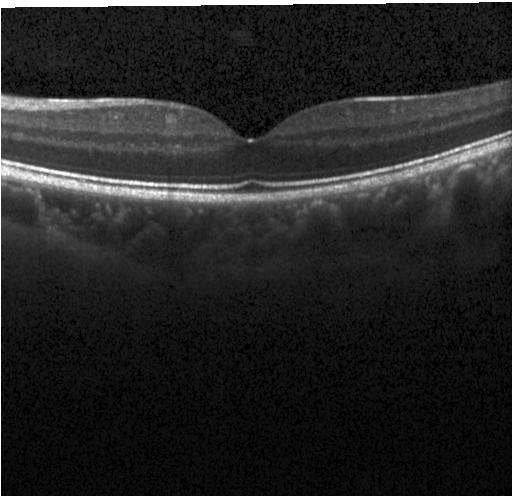

Retinal OCT B-scan
Diagnosis: neither CNV, DME, nor drusen.